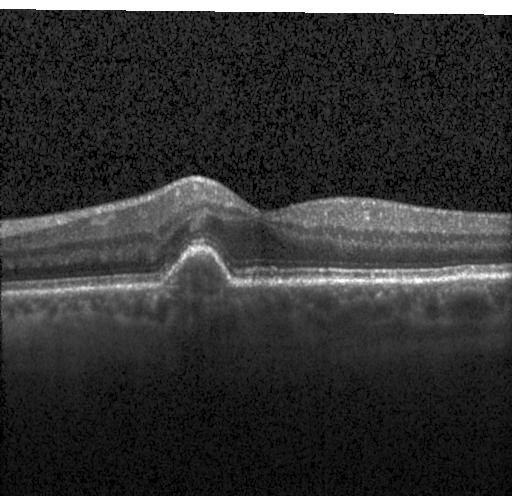 CNV.